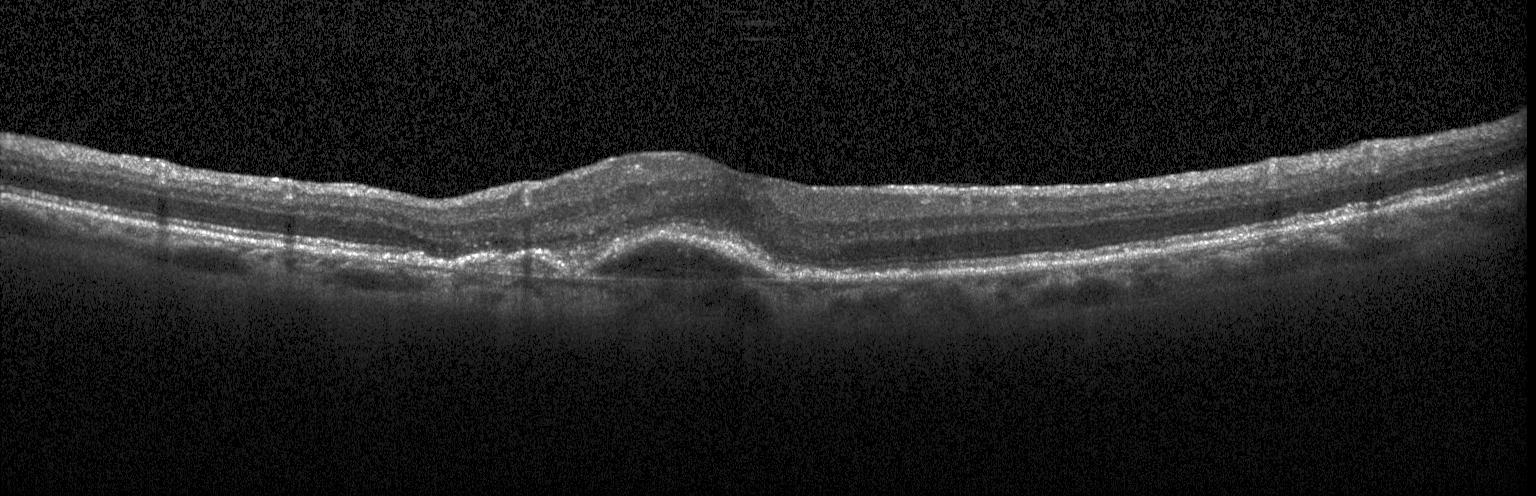 Optical coherence tomography scan.
Finding: choroidal neovascularization.